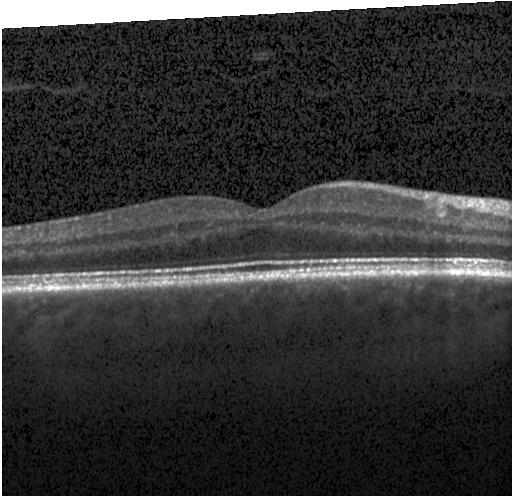 Assessment: neither choroidal neovascularization, diabetic macular edema, nor drusen.